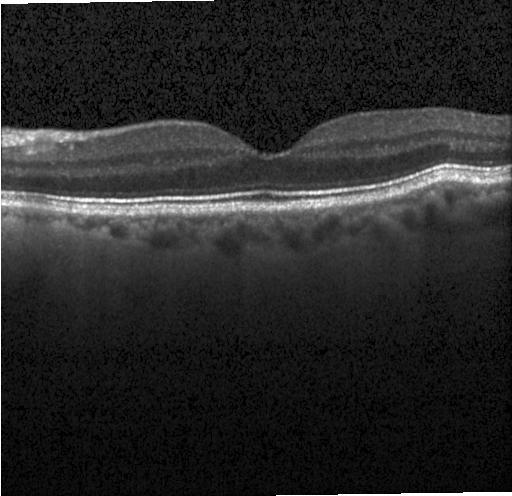 Retinal OCT B-scan; spectral-domain OCT; instrument: Heidelberg Spectralis; horizontal scan through the fovea.
Neither choroidal neovascularization, diabetic macular edema, nor drusen.